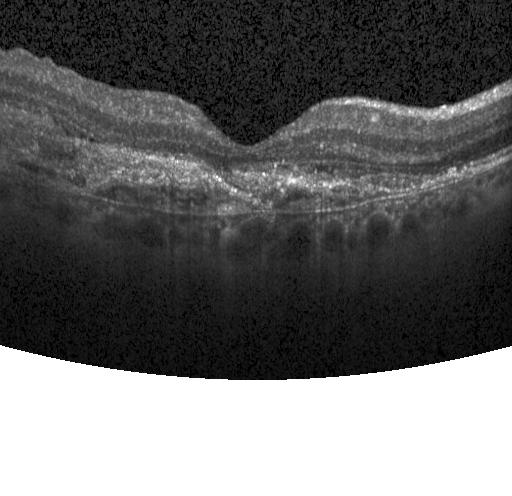

Spectral-domain OCT B-scan: a choroidal neovascular membrane.